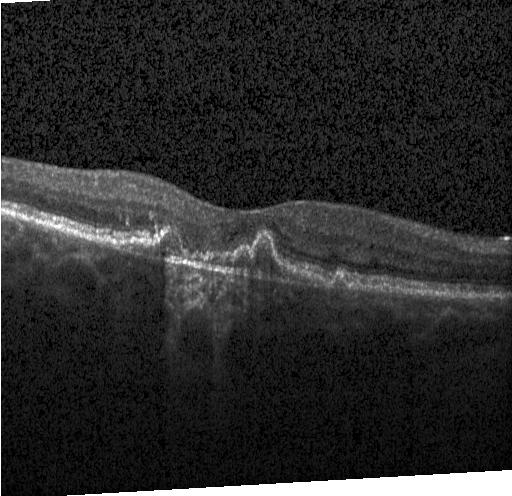 Acquired on a Heidelberg Spectralis; optical coherence tomography scan. OCT finding: a choroidal neovascular membrane.